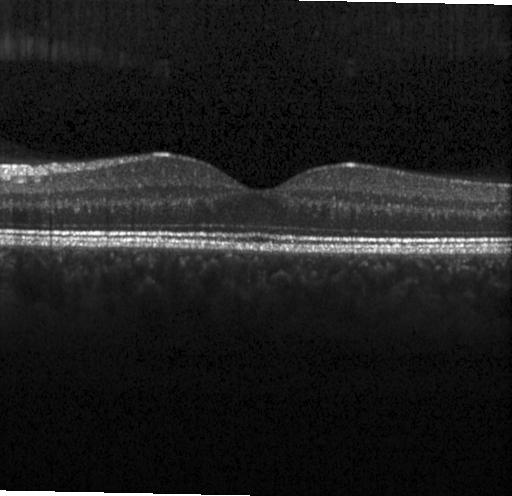
Retinal OCT cross-section · through the macula. Dx: no evidence of choroidal neovascularization, diabetic macular edema, or drusen.